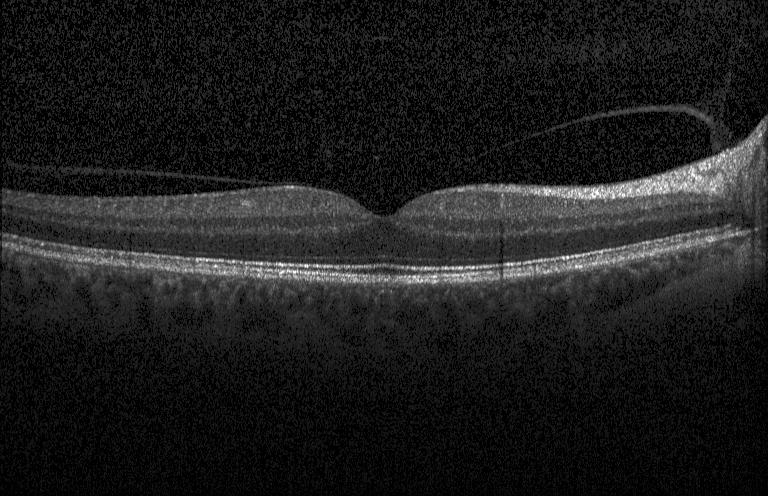 OCT B-scan, spectral-domain optical coherence tomography.
Finding: neither CNV, DME, nor drusen.